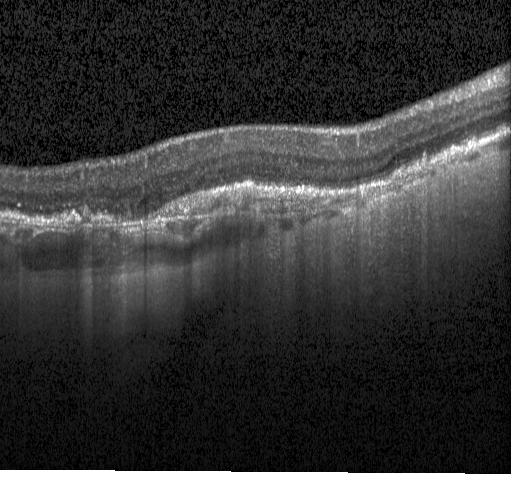 Retinal OCT B-scan · centered on the fovea.
The scan shows a choroidal neovascular membrane.